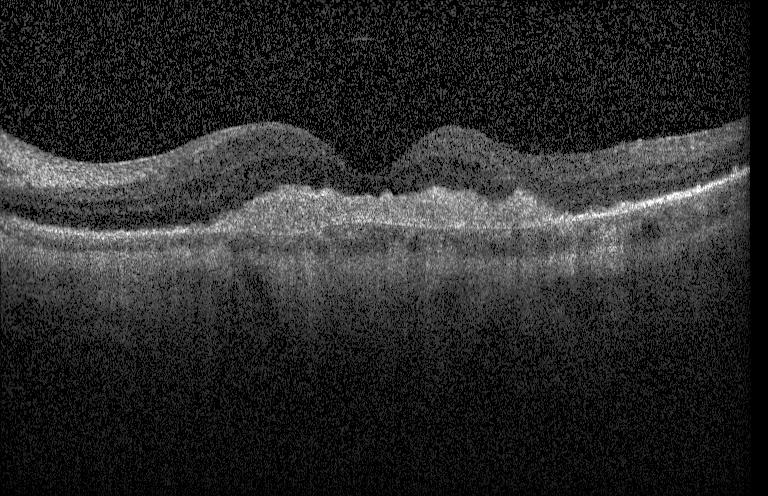
Impression: a choroidal neovascular membrane.